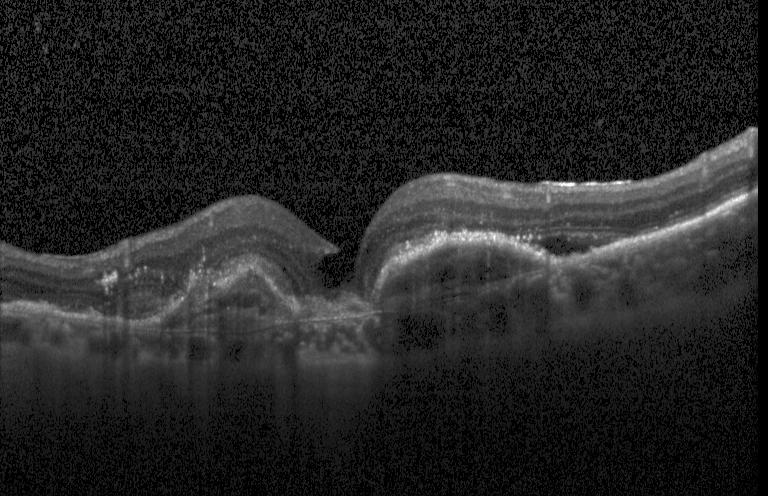 Optical coherence tomography scan · spectral-domain OCT · Heidelberg Spectralis — A choroidal neovascular membrane.